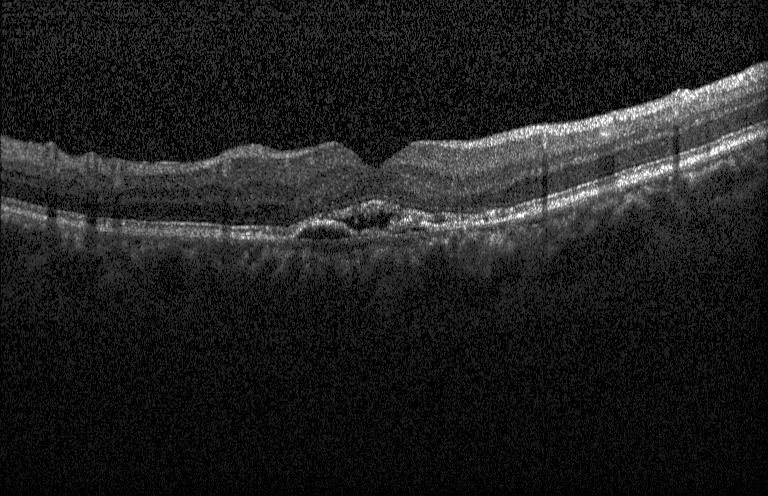 OCT line scan
OCT finding: a choroidal neovascular membrane.